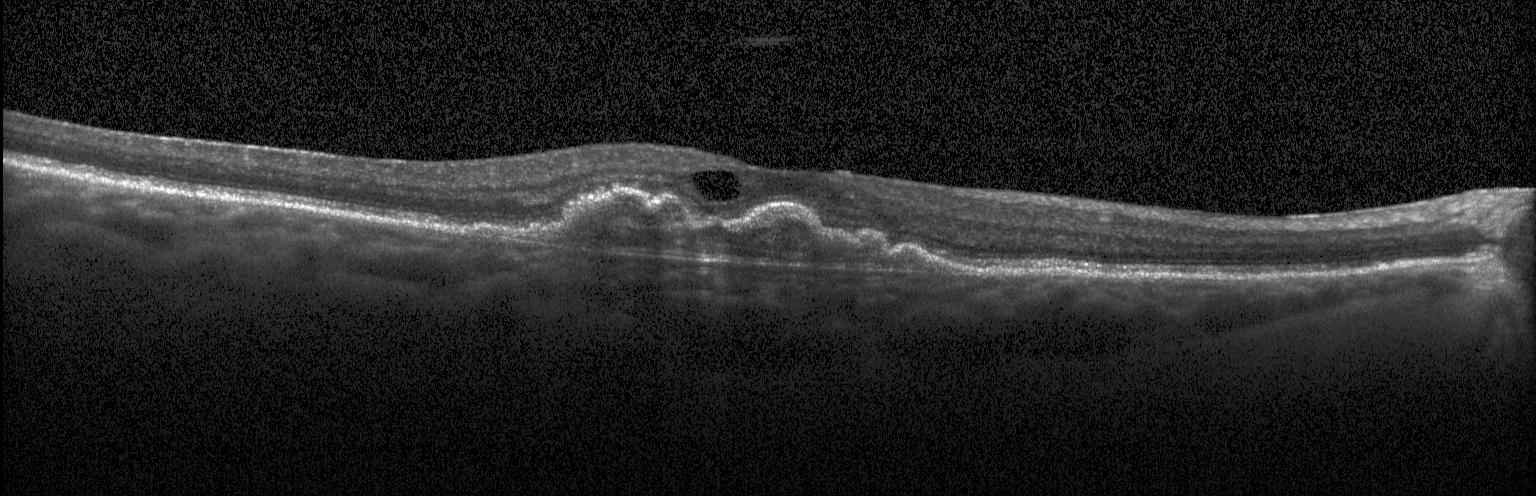

Macular scan, SD-OCT, OCT B-scan — OCT finding: a choroidal neovascular membrane.